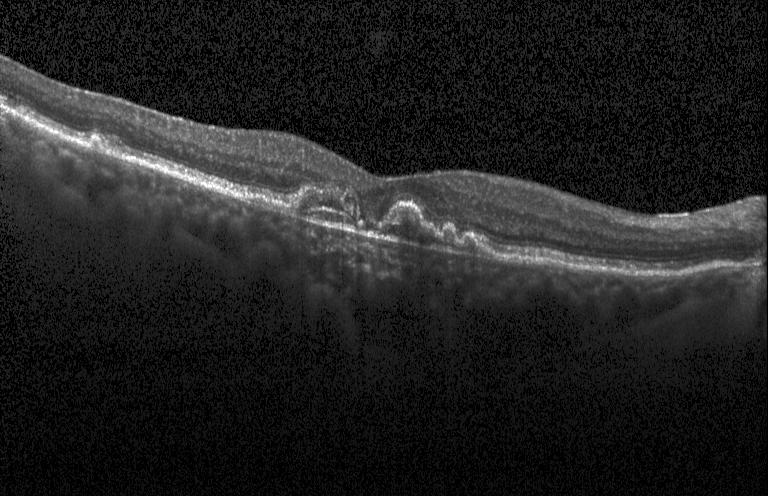

Impression: choroidal neovascularization (CNV).